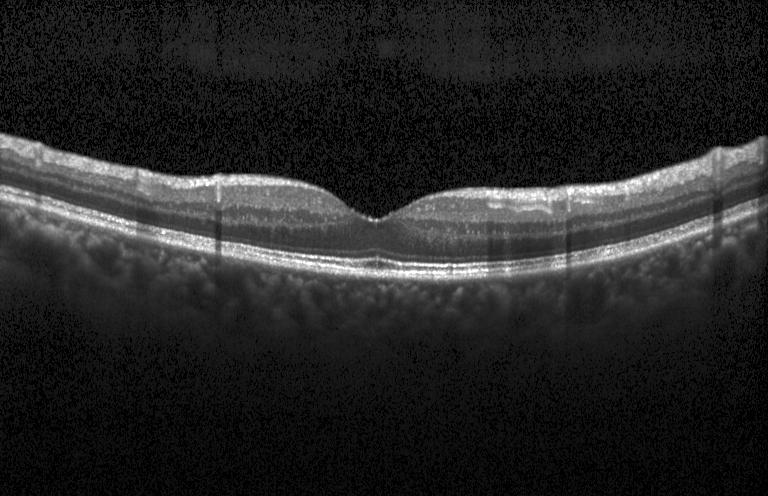
Instrument: Heidelberg Spectralis; SD-OCT; OCT B-scan; through the macula
Dx: no CNV, no DME, and no drusen.